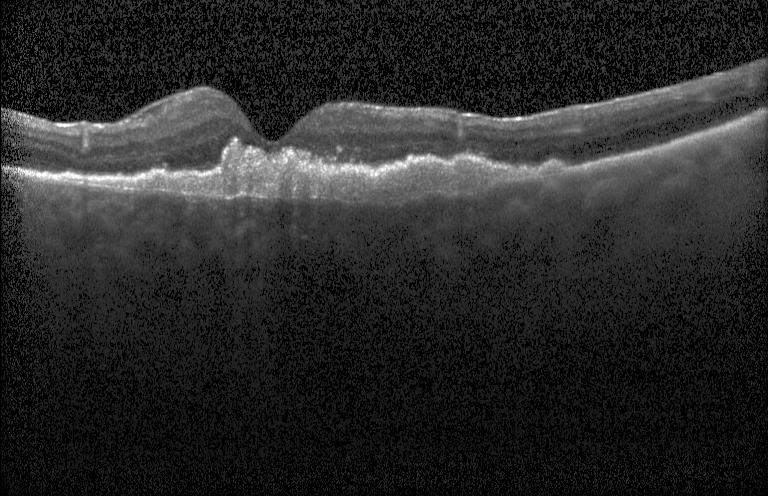 Retinal OCT B-scan. Acquired on a Heidelberg Spectralis.
Finding: a choroidal neovascular membrane.